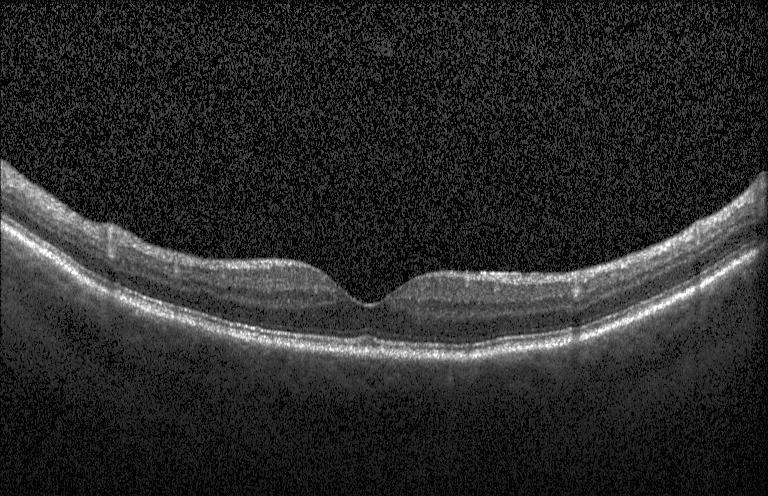 Diagnosis: no choroidal neovascularization, diabetic macular edema, or drusen.